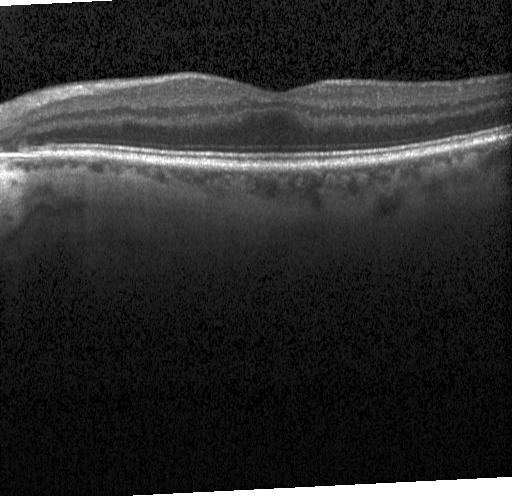 The scan shows no choroidal neovascularization, no diabetic macular edema, and no drusen.